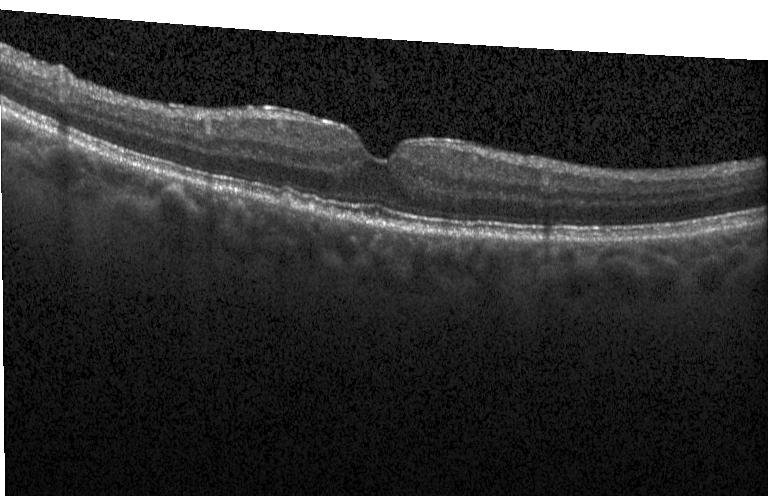
Macular OCT: multiple drusen.